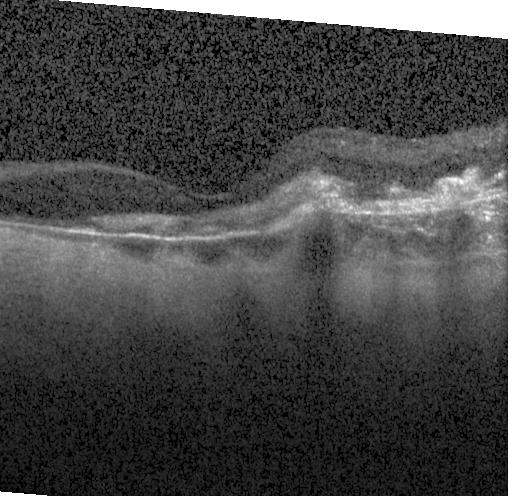 Diagnosis: a choroidal neovascular membrane.